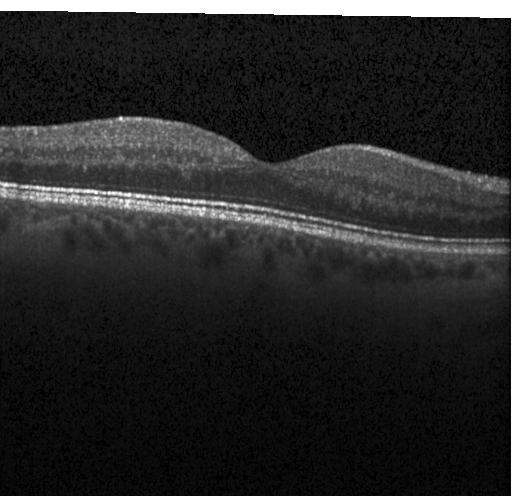

Optical coherence tomography B-scan. Horizontal scan through the fovea. Diagnosis: no choroidal neovascularization, diabetic macular edema, or drusen.